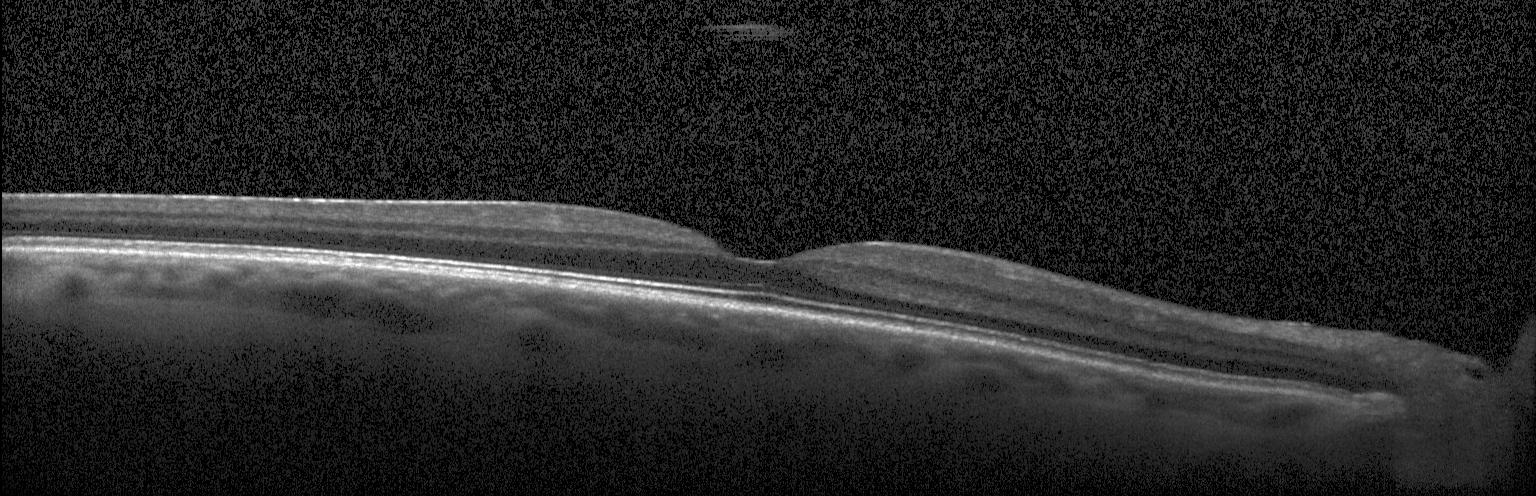
Assessment: no choroidal neovascularization, diabetic macular edema, or drusen.